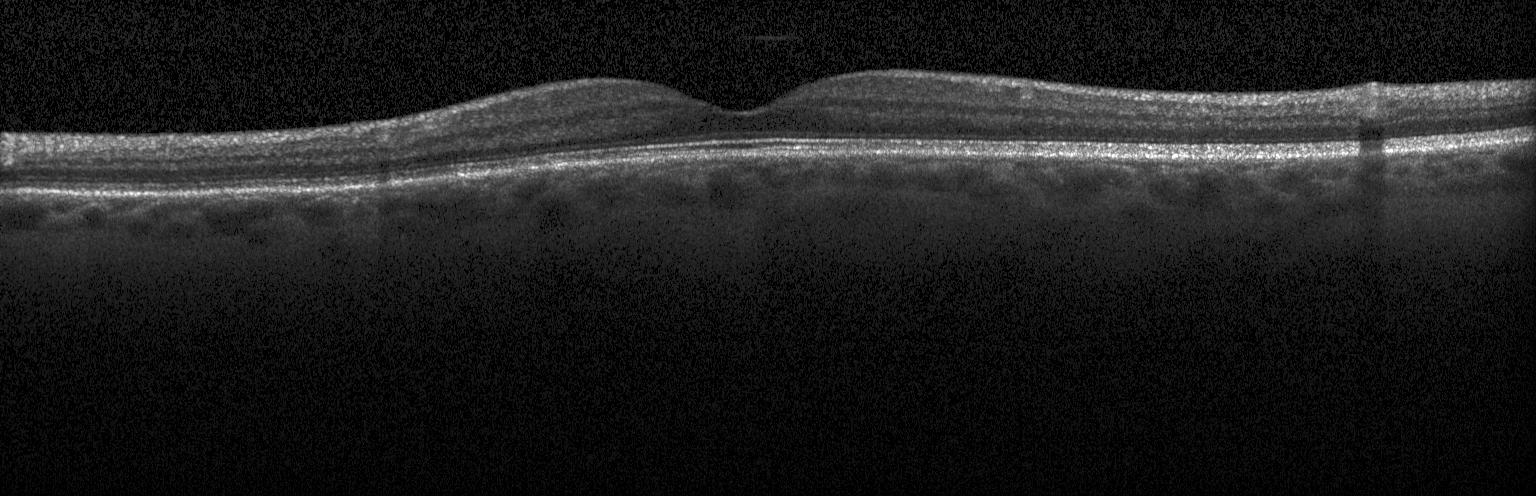 Optical coherence tomography B-scan · spectral-domain optical coherence tomography.
Assessment: no CNV, DME, or drusen.